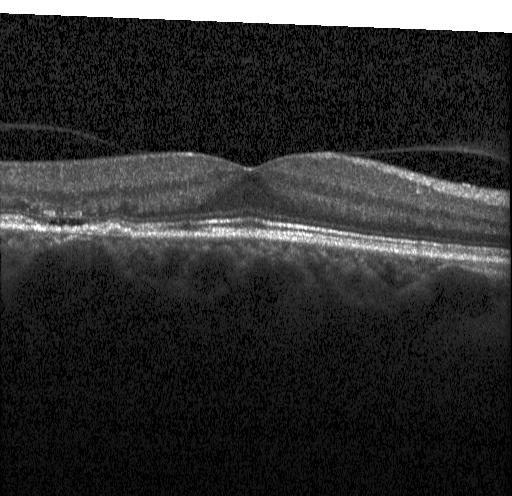

OCT line scan; SD-OCT
Diagnosis: a choroidal neovascular membrane.